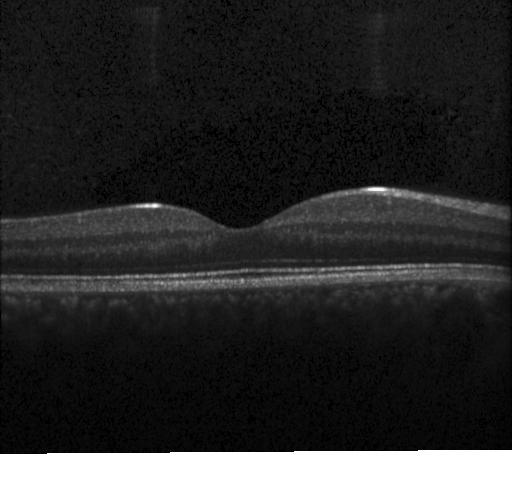
Fovea-centered · spectral-domain OCT · retinal OCT cross-section · instrument: Heidelberg Spectralis
This B-scan demonstrates no choroidal neovascularization, diabetic macular edema, or drusen.